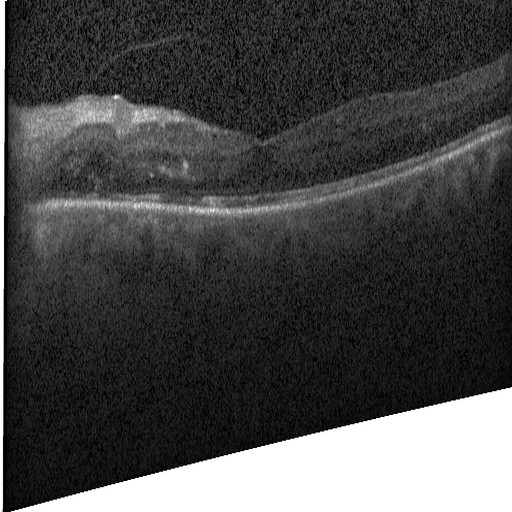 Heidelberg Spectralis, fovea-centered, spectral-domain OCT, OCT line scan. Impression: diabetic macular edema.